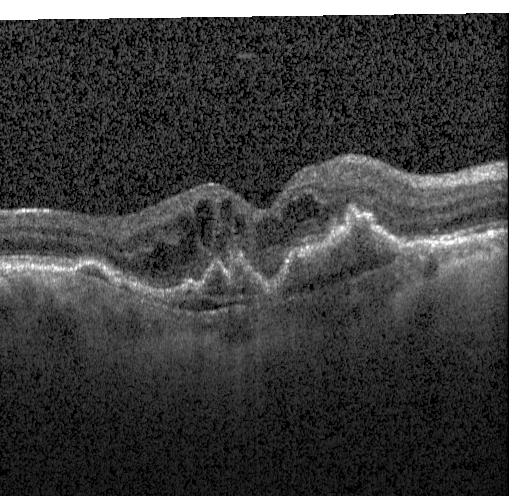
Heidelberg Spectralis; OCT line scan; centered on the fovea; spectral-domain optical coherence tomography.
A choroidal neovascular membrane.